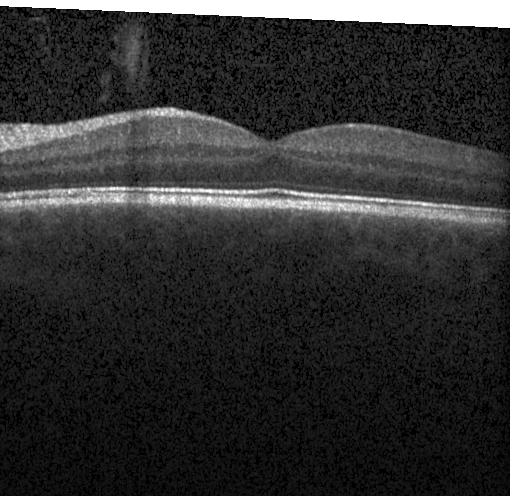 The scan shows no CNV, no DME, and no drusen.